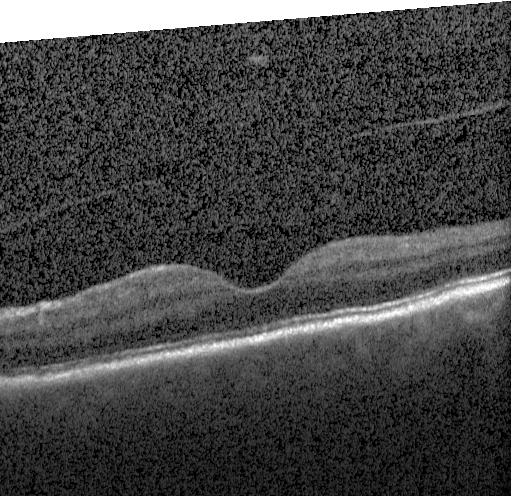

Heidelberg Spectralis; SD-OCT; retinal OCT B-scan.
Diagnosis: no CNV, no DME, and no drusen.